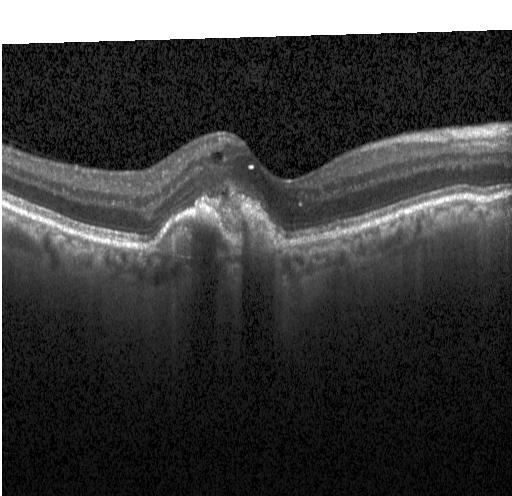

Diagnosis: a choroidal neovascular membrane.